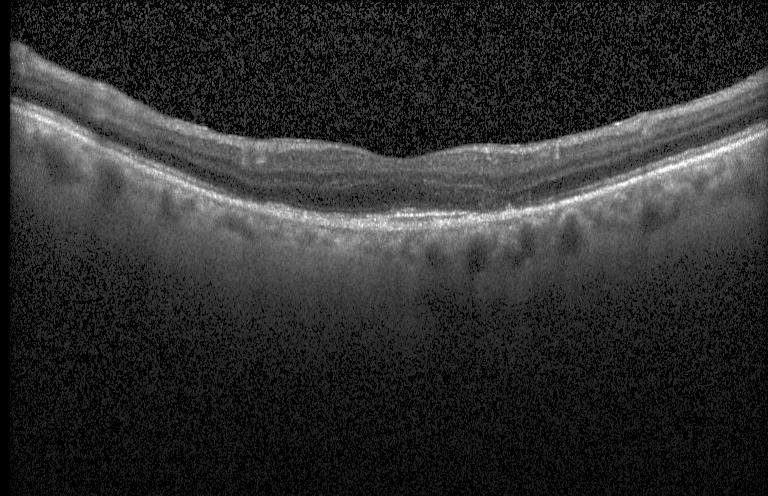 Spectral-domain optical coherence tomography. Optical coherence tomography scan. Instrument: Heidelberg Spectralis
Assessment: a choroidal neovascular membrane.